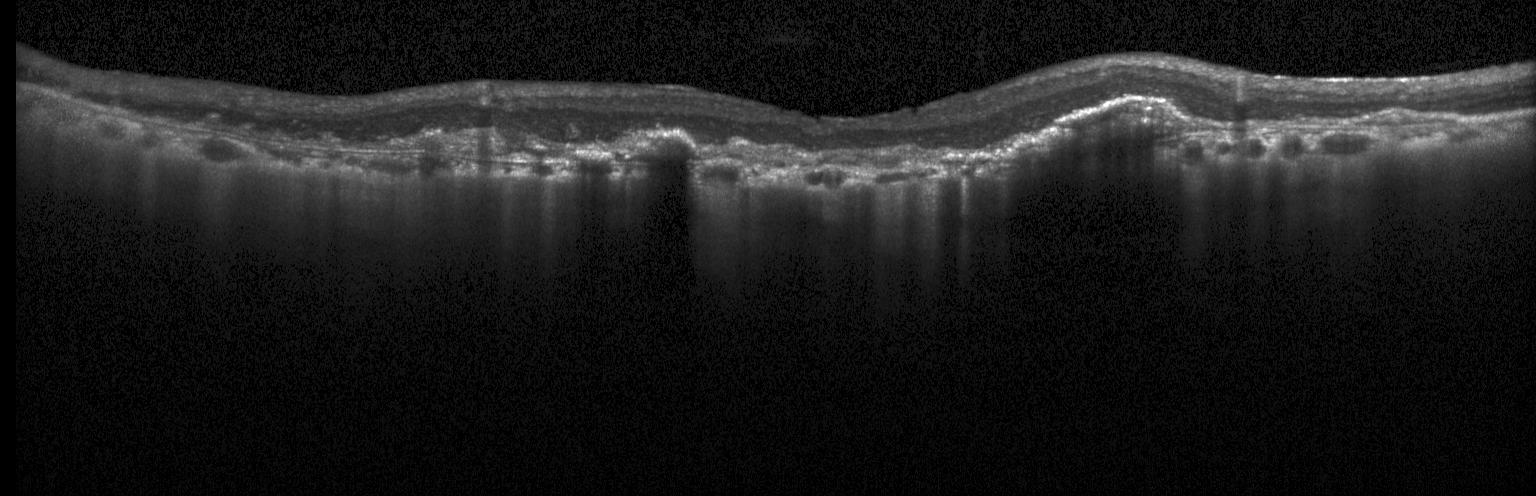 Assessment: choroidal neovascularization.